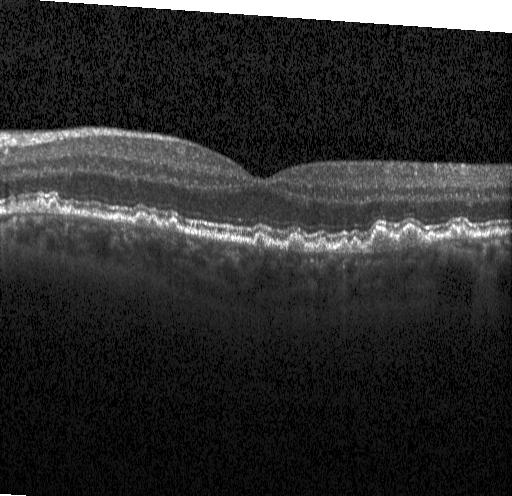

OCT scan showing sub-RPE drusenoid deposits.